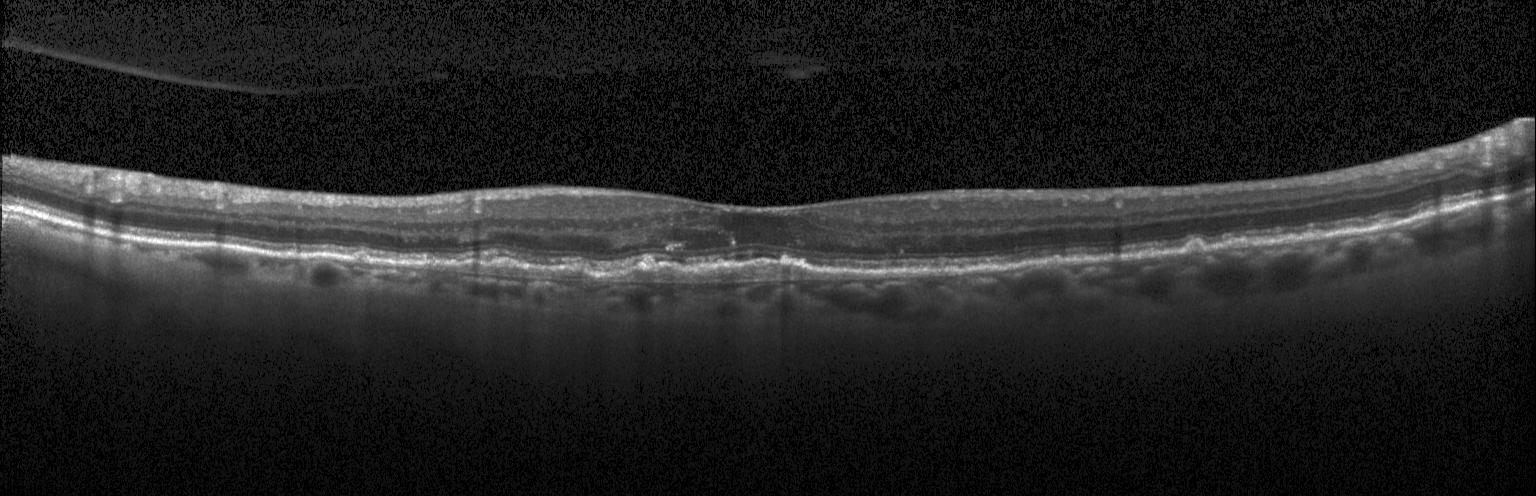
Retinal OCT cross-section
The scan shows a choroidal neovascular membrane.